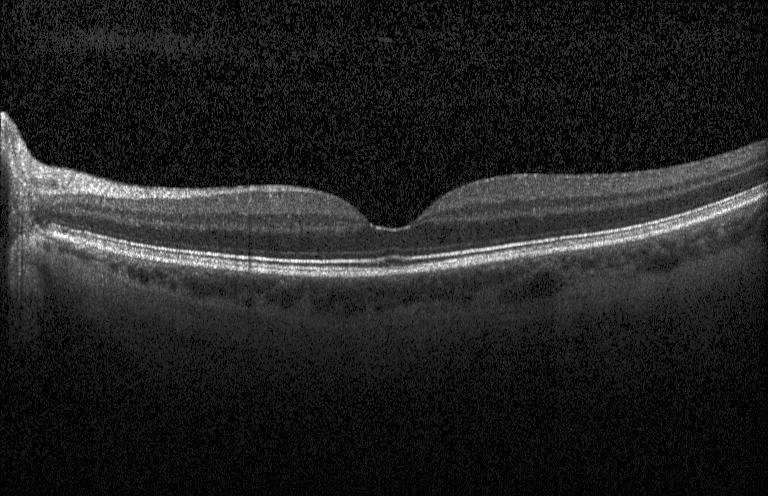
OCT scan showing neither choroidal neovascularization, diabetic macular edema, nor drusen.